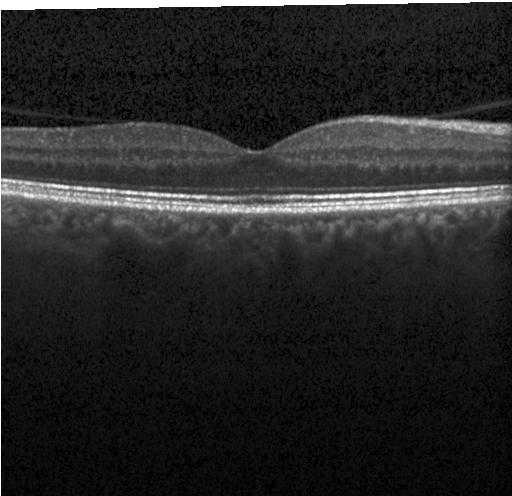
Horizontal scan through the fovea · spectral-domain OCT · optical coherence tomography scan · instrument: Heidelberg Spectralis.
Diagnosis: no CNV, DME, or drusen.